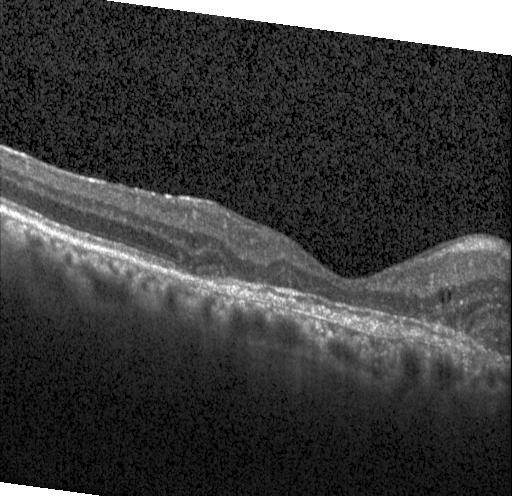
Spectral-domain OCT. Retinal OCT cross-section.
OCT finding: choroidal neovascularization.